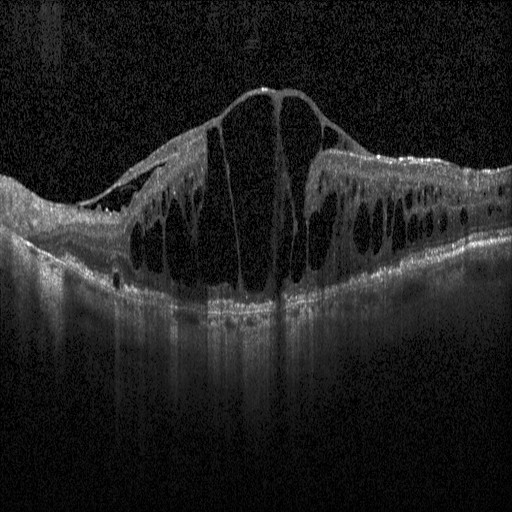
Optical coherence tomography scan, spectral-domain OCT, macular scan.
This B-scan demonstrates DME.